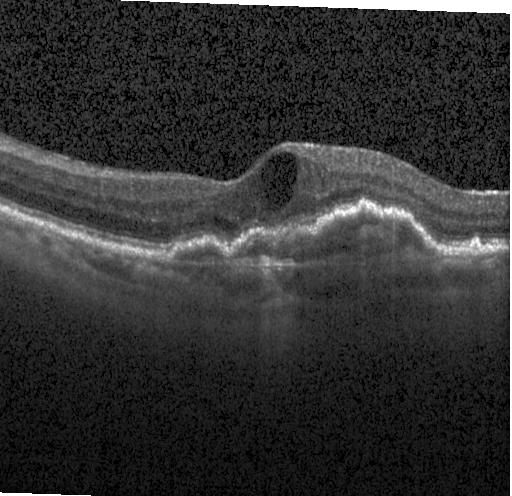 Macular OCT: a choroidal neovascular membrane.